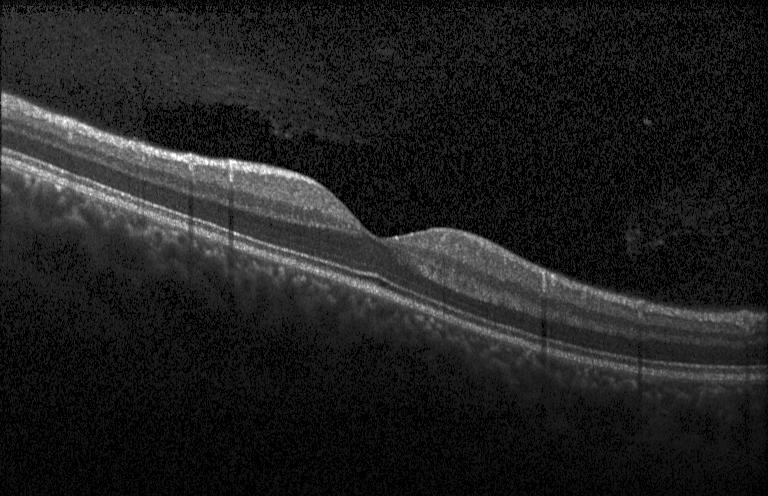 Spectral-domain OCT; through the macula; retinal OCT cross-section; Heidelberg Spectralis.
No choroidal neovascularization, diabetic macular edema, or drusen.